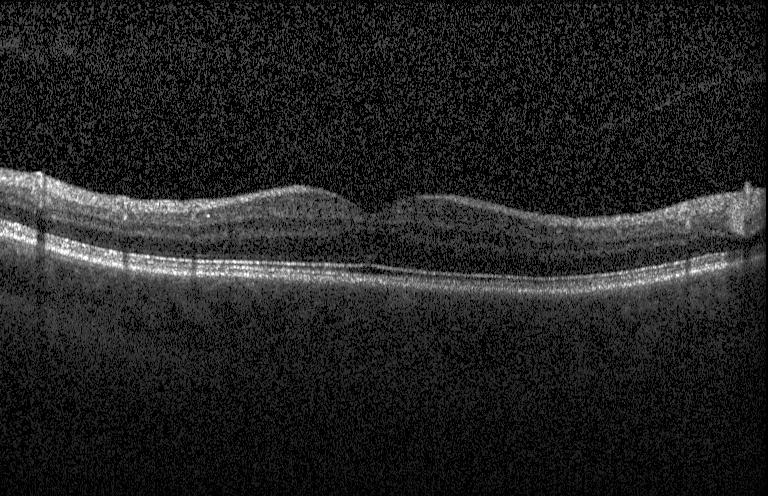
Instrument: Heidelberg Spectralis · optical coherence tomography scan. Finding: no choroidal neovascularization, diabetic macular edema, or drusen.